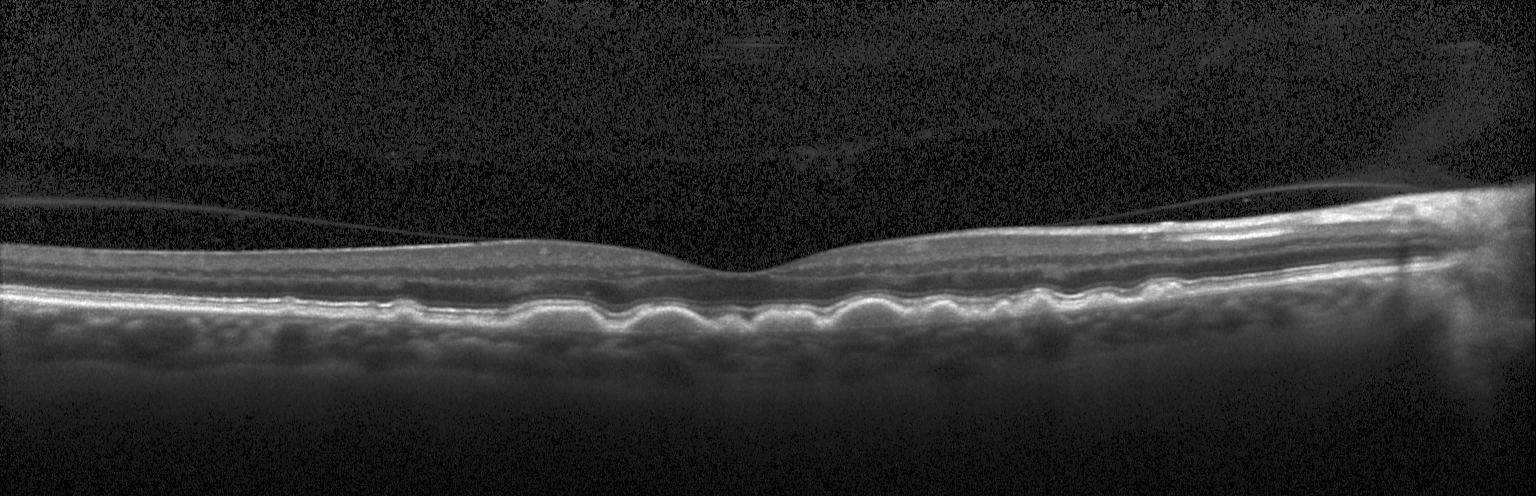
Heidelberg Spectralis OCT system · retinal OCT cross-section · fovea-centered — Assessment: sub-RPE drusenoid deposits.